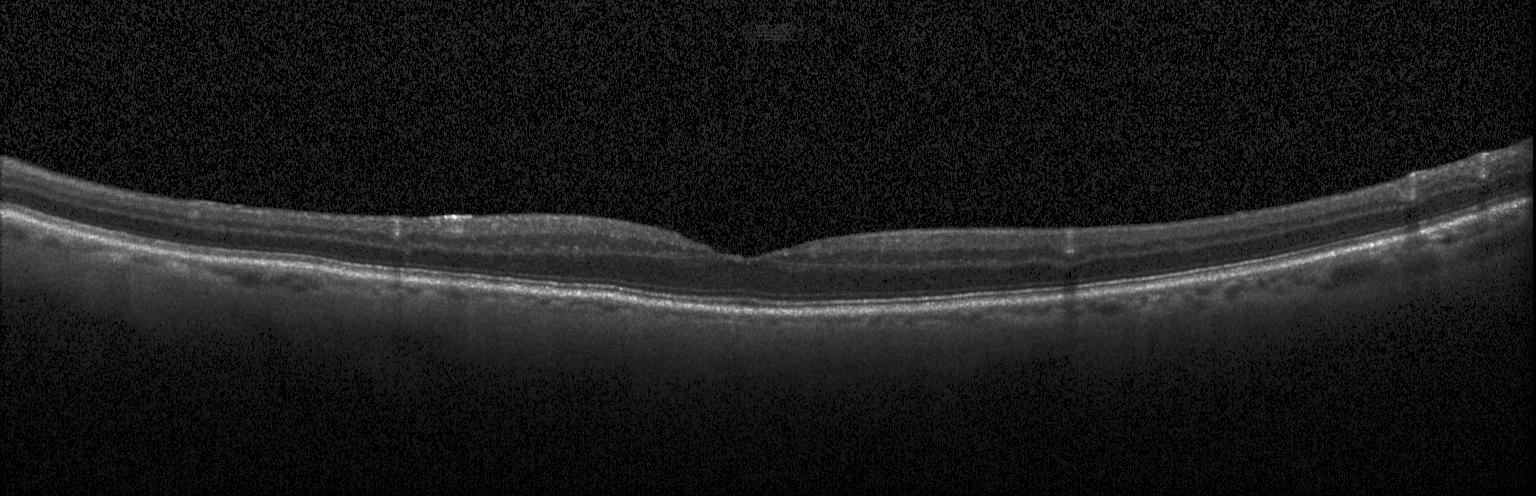 OCT B-scan.
The scan shows neither CNV, DME, nor drusen.